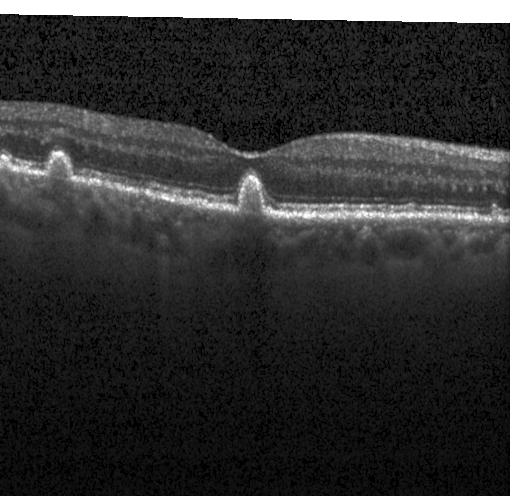
Assessment: multiple drusen.